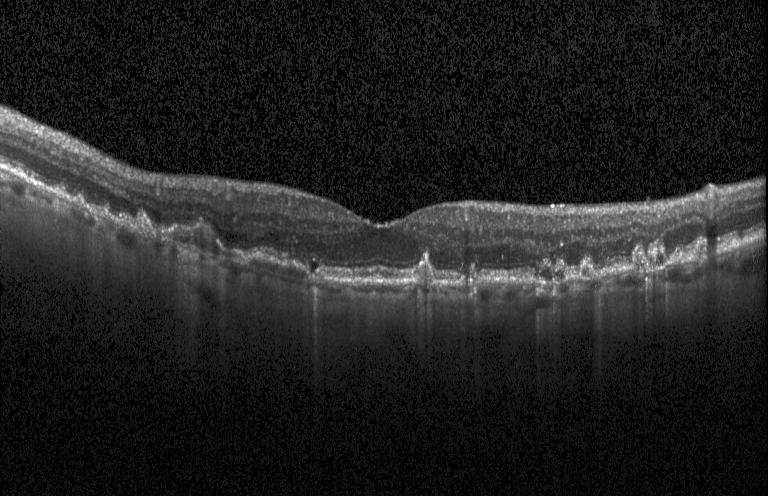
Diagnosis: a choroidal neovascular membrane.